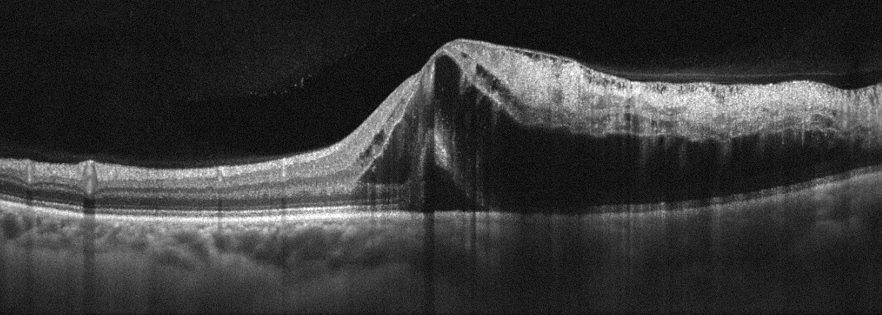 Impression: retinal vein occlusion.